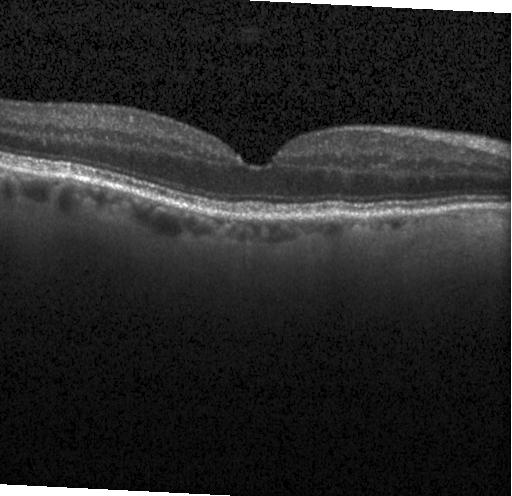

Spectral-domain OCT. Macular scan. Heidelberg Spectralis OCT system. Retinal OCT B-scan — OCT finding: neither choroidal neovascularization, diabetic macular edema, nor drusen.